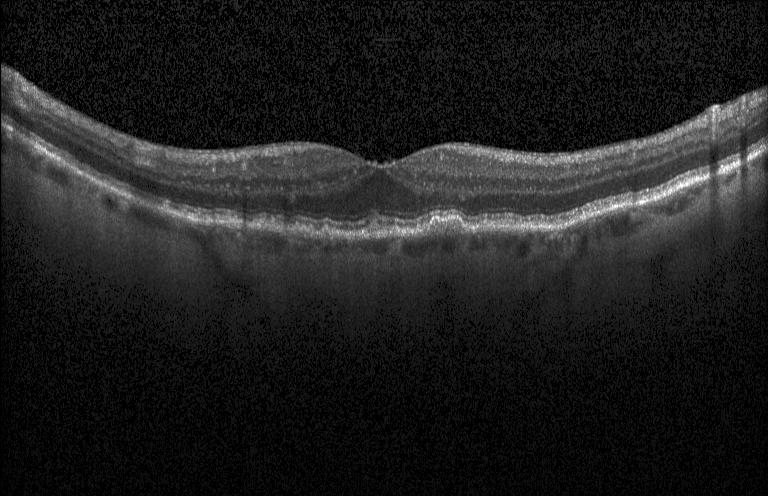

Retinal OCT cross-section showing sub-RPE drusenoid deposits.